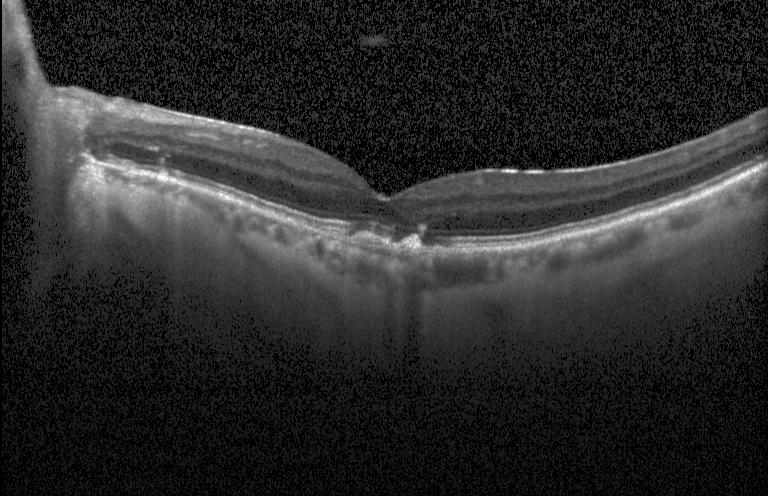 Centered on the fovea, OCT B-scan, Heidelberg Spectralis. Impression: a choroidal neovascular membrane.